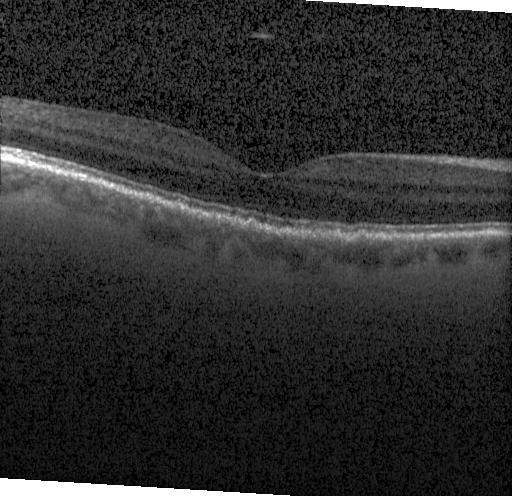 Impression: multiple drusen.